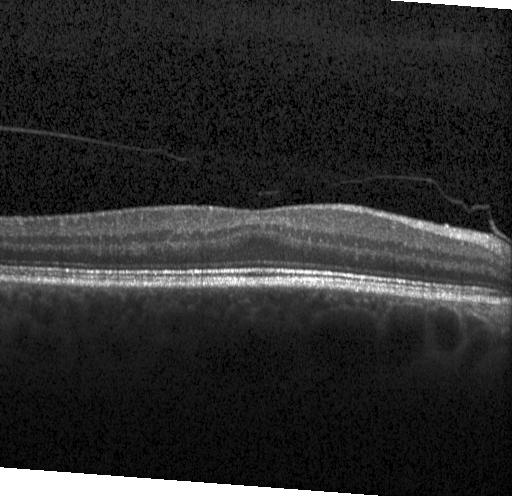
Retinal OCT cross-section. This B-scan demonstrates neither CNV, DME, nor drusen.